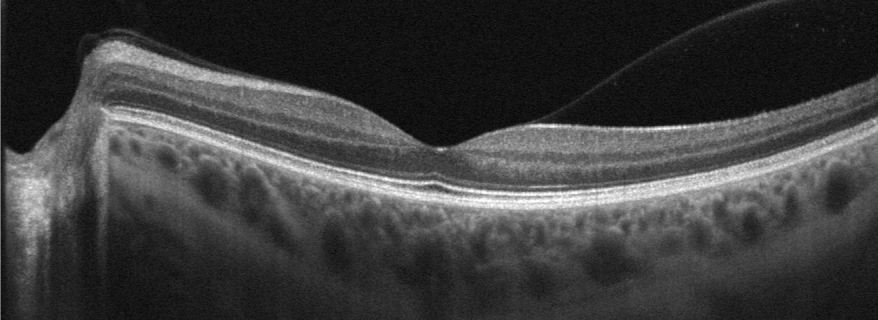
Optovue Avanti RTVue XR · retinal OCT B-scan
Impression: no evidence of AMD, DME, ERM, RAO, RVO, or VID.